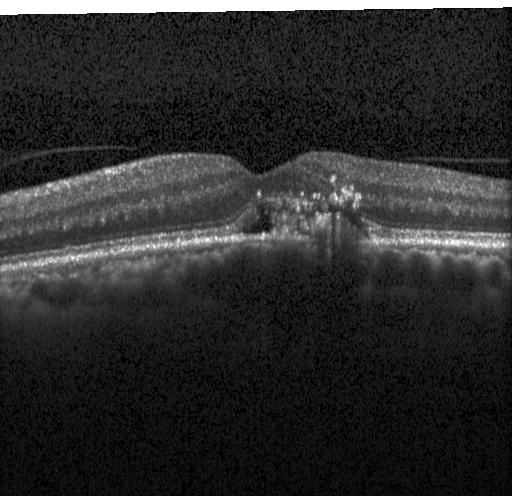
SD-OCT. Fovea-centered. Acquired on a Heidelberg Spectralis. Optical coherence tomography scan — Diagnosis: a choroidal neovascular membrane.